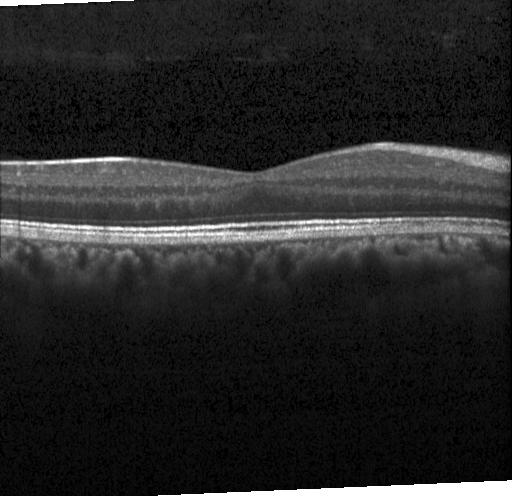
Instrument: Heidelberg Spectralis. OCT line scan. Spectral-domain OCT
Impression: no choroidal neovascularization, diabetic macular edema, or drusen.